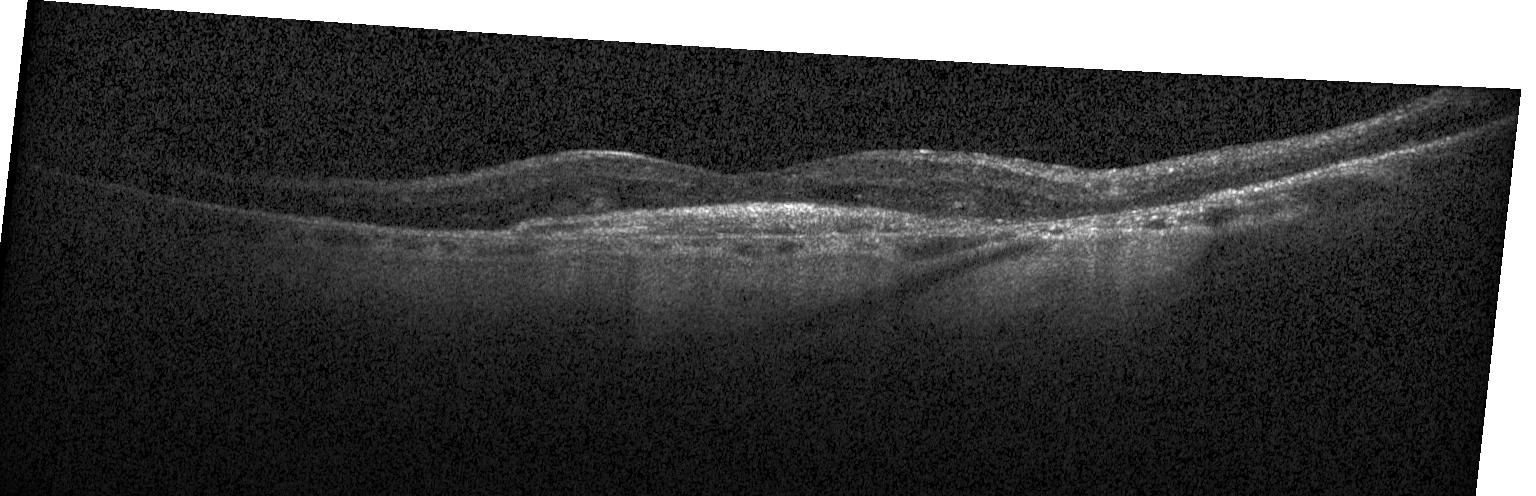

SD-OCT, OCT B-scan
Finding: a choroidal neovascular membrane.